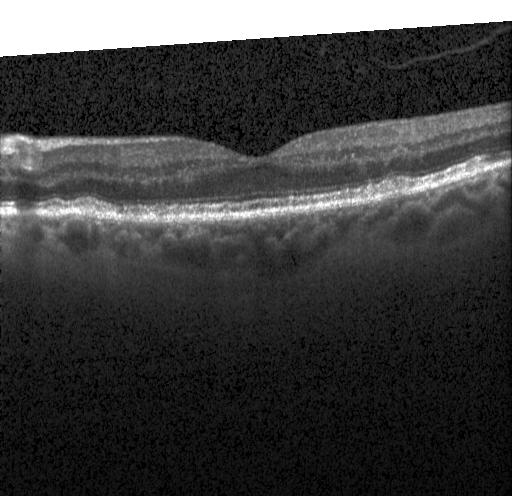 Fovea-centered; retinal OCT B-scan; Heidelberg Spectralis OCT system; spectral-domain OCT — Impression: drusen.